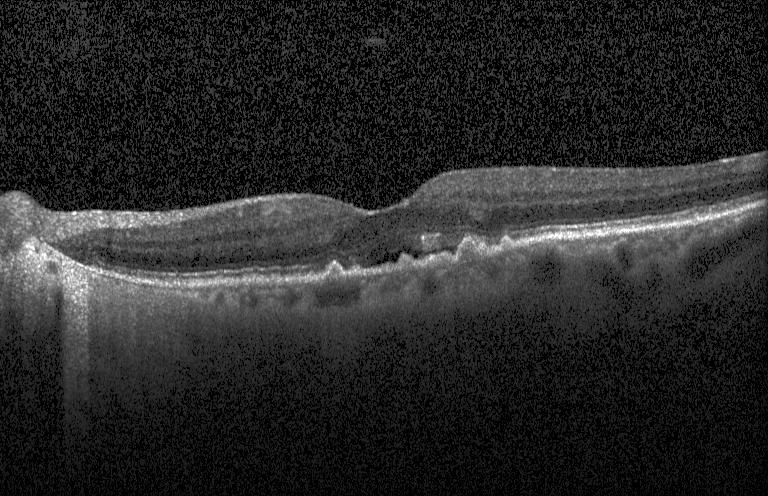 Finding: choroidal neovascularization (CNV).